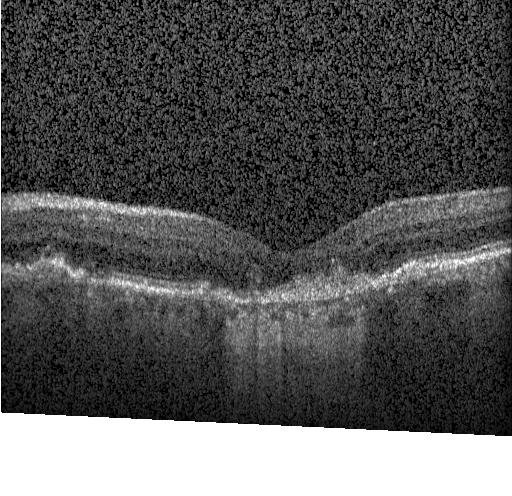 Instrument: Heidelberg Spectralis, retinal OCT cross-section — Finding: a choroidal neovascular membrane.